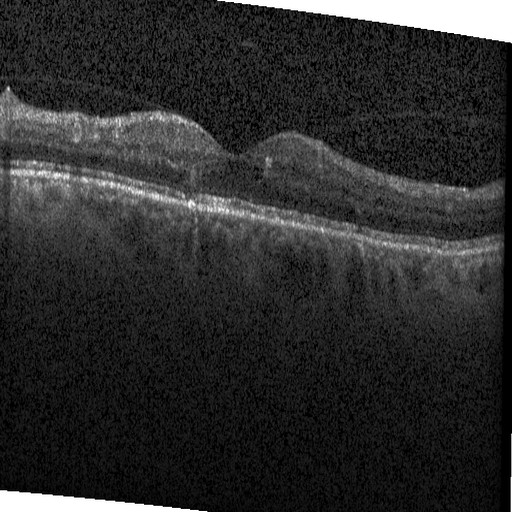

Finding: diabetic macular edema.